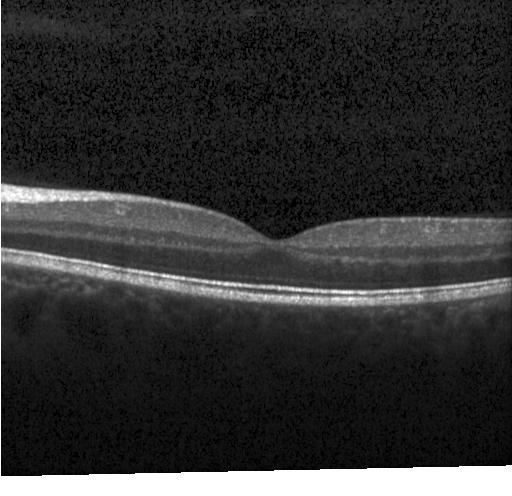 Acquired on a Heidelberg Spectralis; centered on the fovea; SD-OCT; OCT B-scan — Dx: no CNV, no DME, and no drusen.